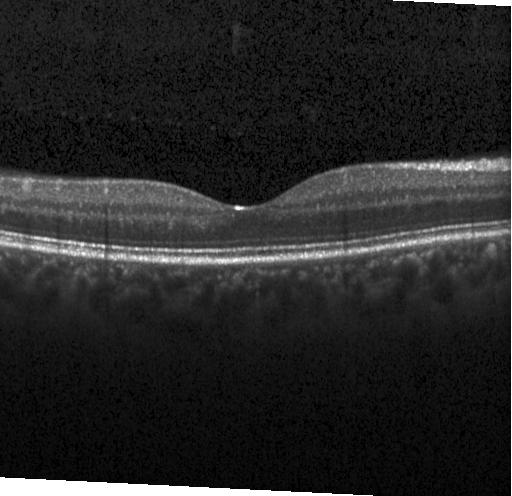

Optical coherence tomography scan. Spectral-domain optical coherence tomography. Heidelberg Spectralis OCT system — This B-scan demonstrates no evidence of choroidal neovascularization, diabetic macular edema, or drusen.